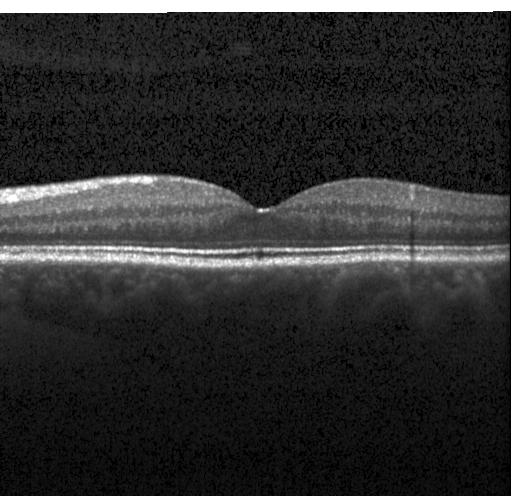
Optical coherence tomography B-scan; acquired on a Heidelberg Spectralis — OCT finding: no choroidal neovascularization, diabetic macular edema, or drusen.